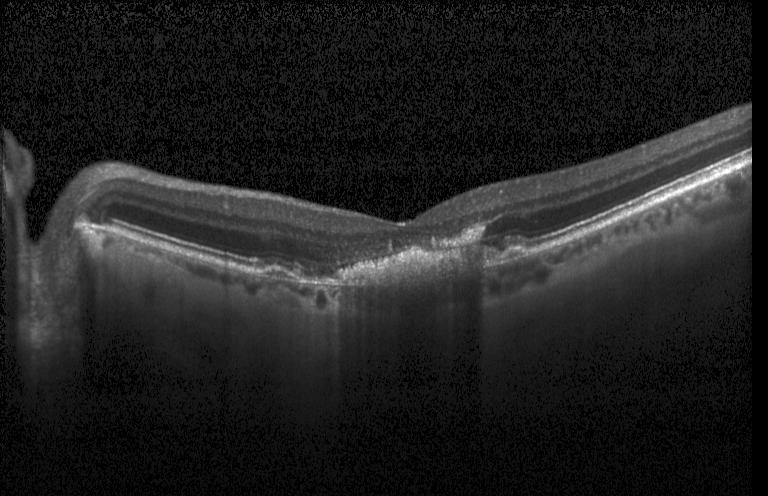
Macular OCT demonstrating CNV.